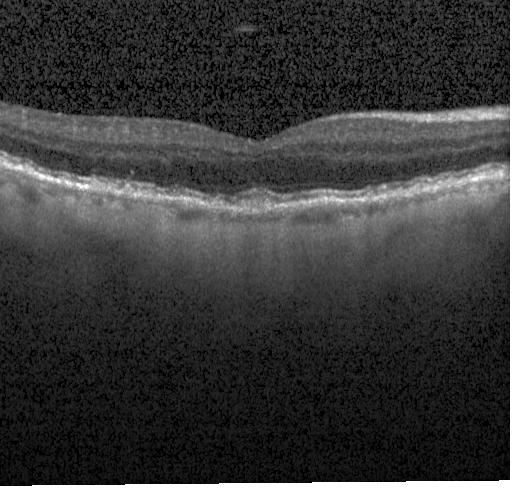

OCT finding: drusen.